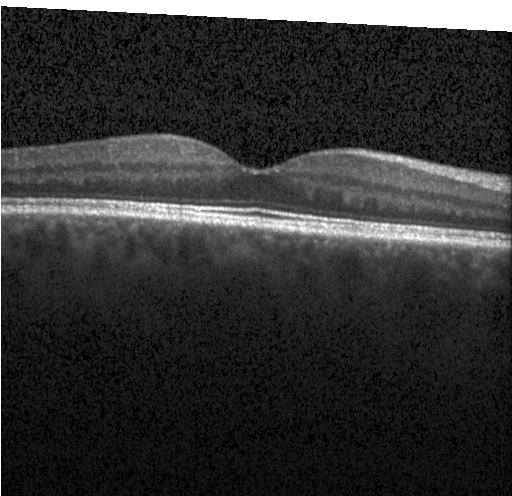

Optical coherence tomography B-scan. This B-scan demonstrates neither choroidal neovascularization, diabetic macular edema, nor drusen.